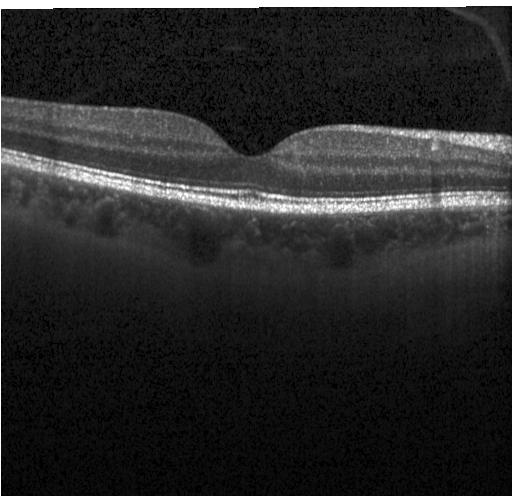

Heidelberg Spectralis, SD-OCT, OCT B-scan
Impression: no choroidal neovascularization, diabetic macular edema, or drusen.